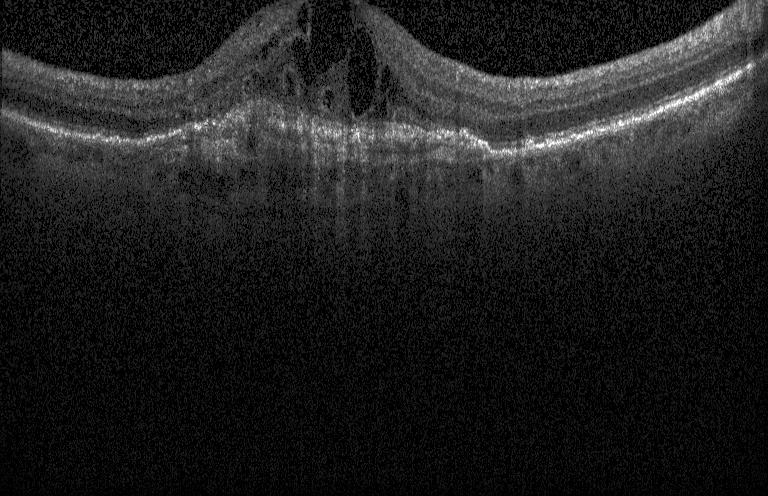

Retinal OCT cross-section showing choroidal neovascularization.